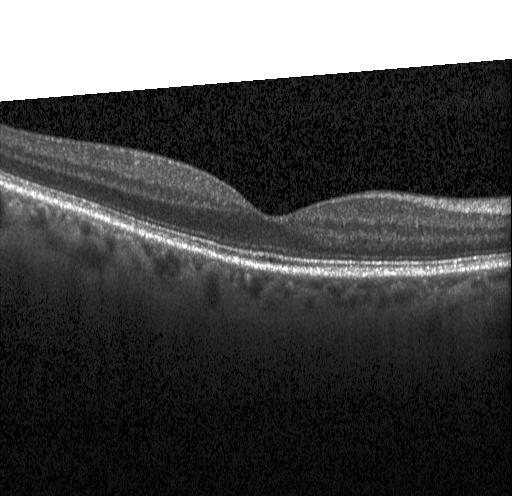

This B-scan demonstrates no choroidal neovascularization, no diabetic macular edema, and no drusen.